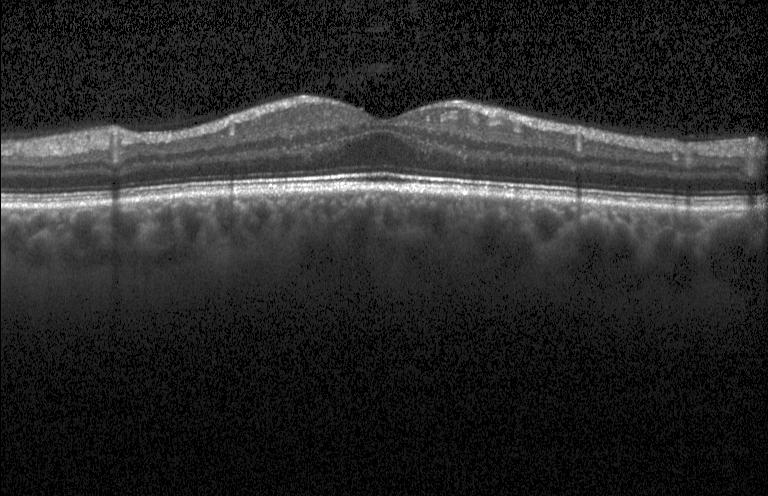
Through the macula, instrument: Heidelberg Spectralis, SD-OCT, optical coherence tomography B-scan — Finding: no evidence of choroidal neovascularization, diabetic macular edema, or drusen.